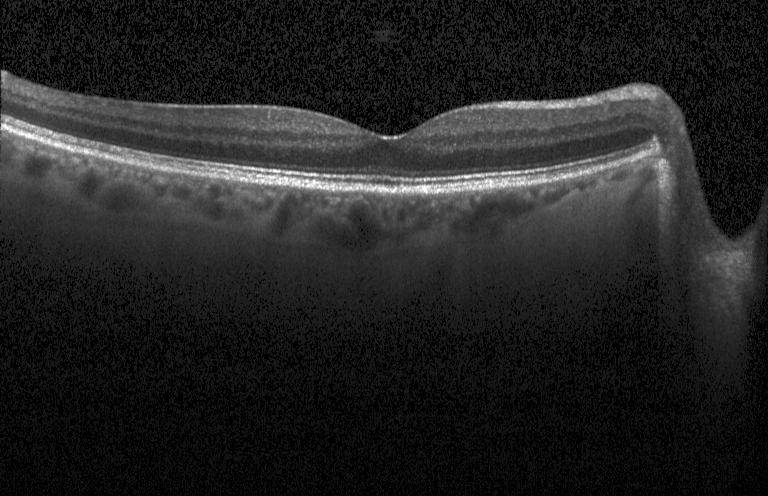

Retinal OCT cross-section
Assessment: no choroidal neovascularization, no diabetic macular edema, and no drusen.